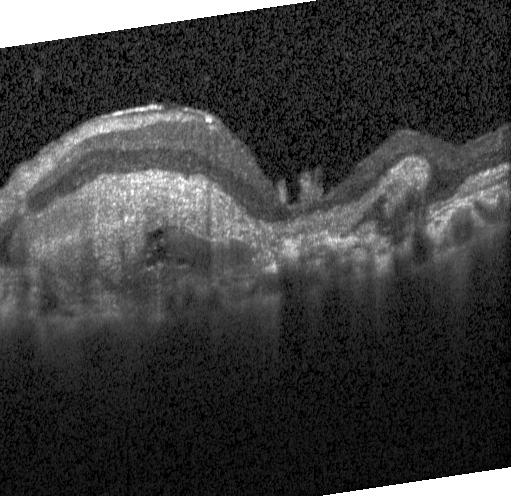
Choroidal neovascularization.